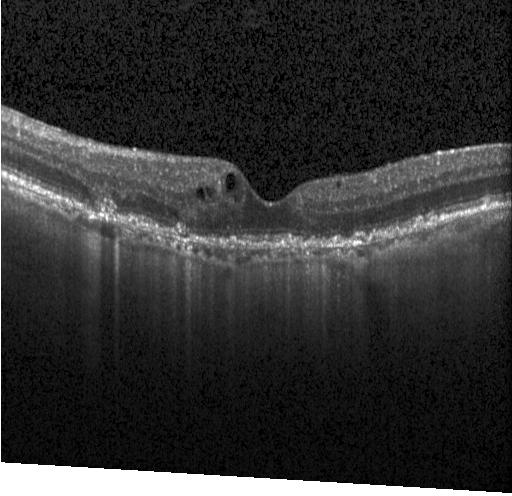

OCT line scan
This B-scan demonstrates a choroidal neovascular membrane.